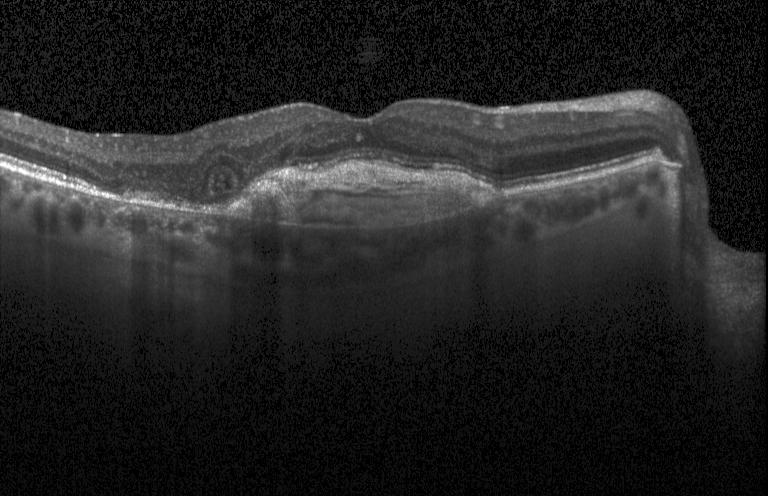 Optical coherence tomography scan.
Assessment: CNV.